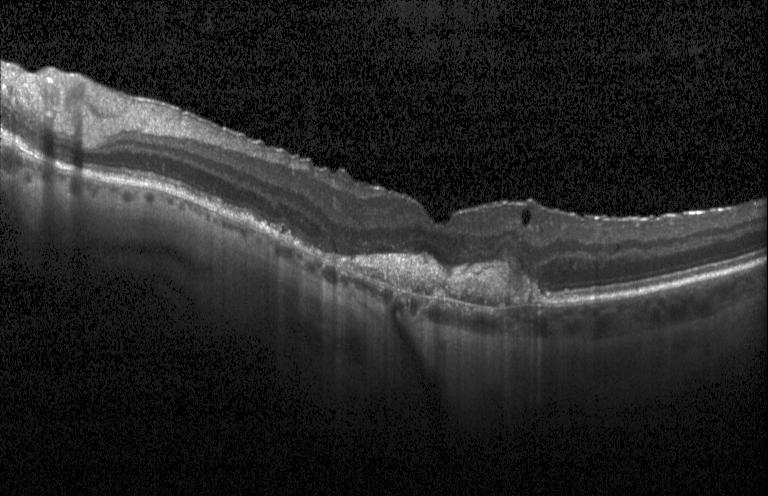
Diagnosis: a choroidal neovascular membrane.